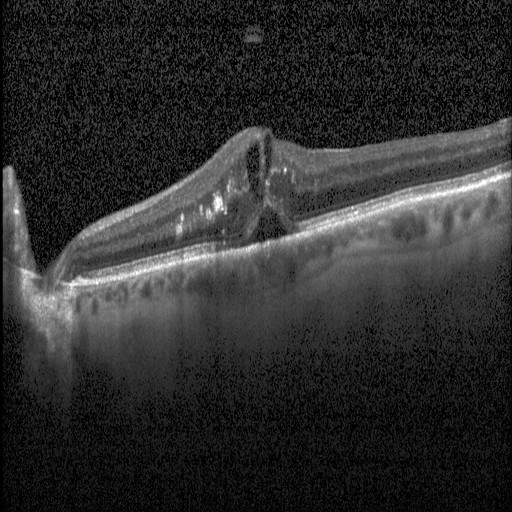 This B-scan demonstrates diabetic macular edema (DME).